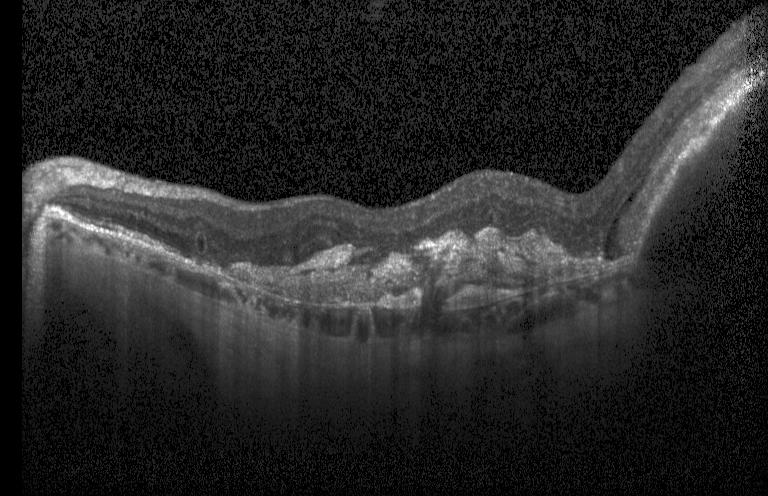

OCT line scan.
Dx: a choroidal neovascular membrane.